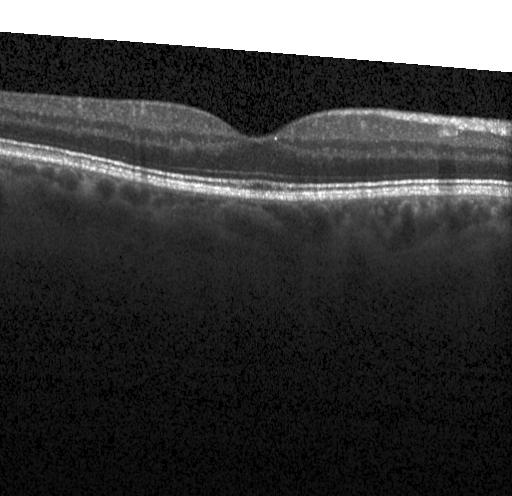

OCT line scan. This B-scan demonstrates no choroidal neovascularization, diabetic macular edema, or drusen.